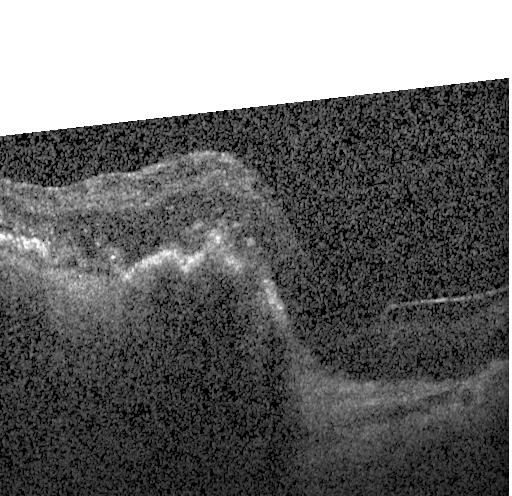 Heidelberg Spectralis; through the macula; optical coherence tomography scan; spectral-domain OCT. Assessment: a choroidal neovascular membrane.